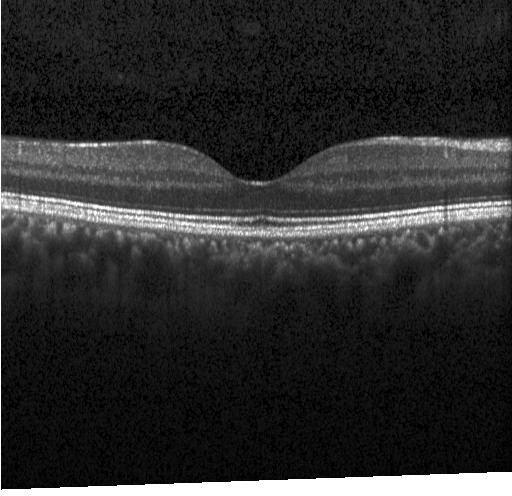 OCT finding: neither choroidal neovascularization, diabetic macular edema, nor drusen.